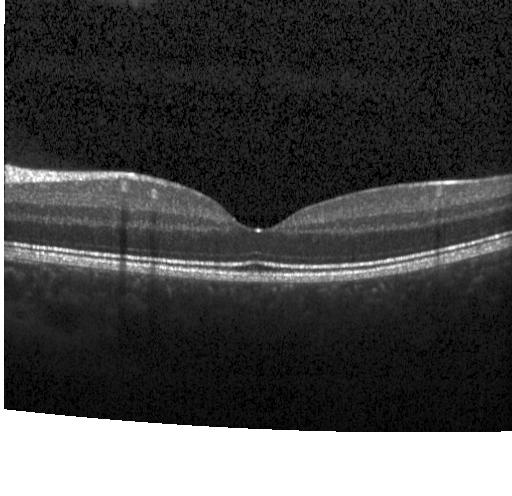

OCT line scan. No evidence of choroidal neovascularization, diabetic macular edema, or drusen.